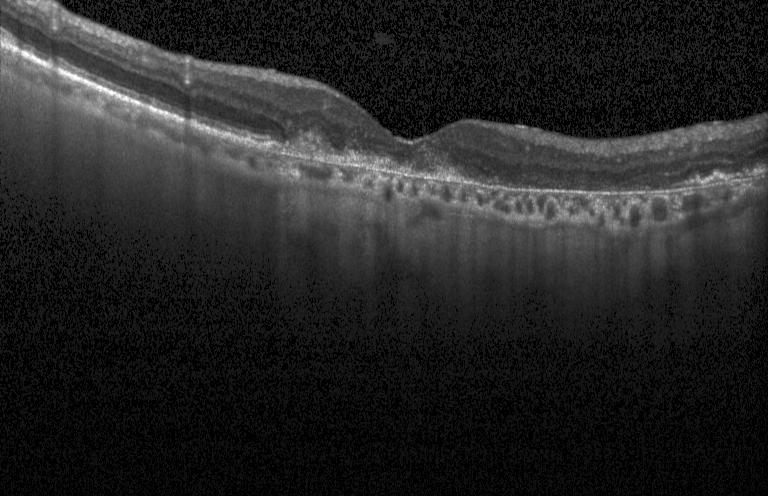 Instrument: Heidelberg Spectralis. Optical coherence tomography scan. Spectral-domain optical coherence tomography. Through the macula. This B-scan demonstrates a choroidal neovascular membrane.